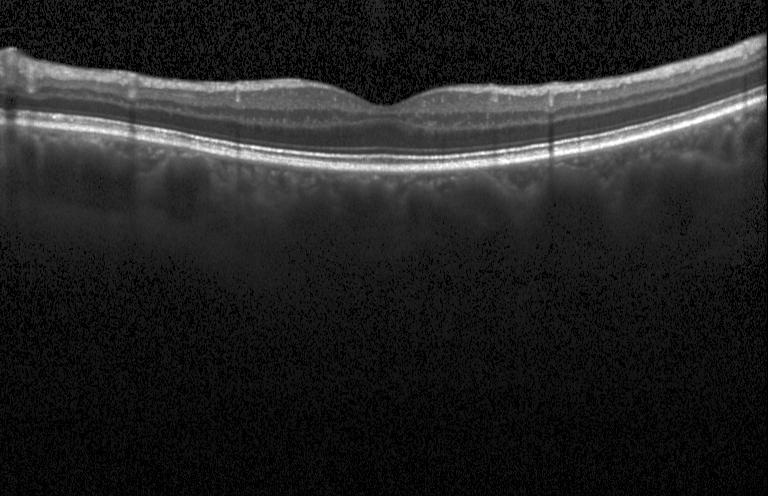
Optical coherence tomography B-scan. Diagnosis: no CNV, DME, or drusen.